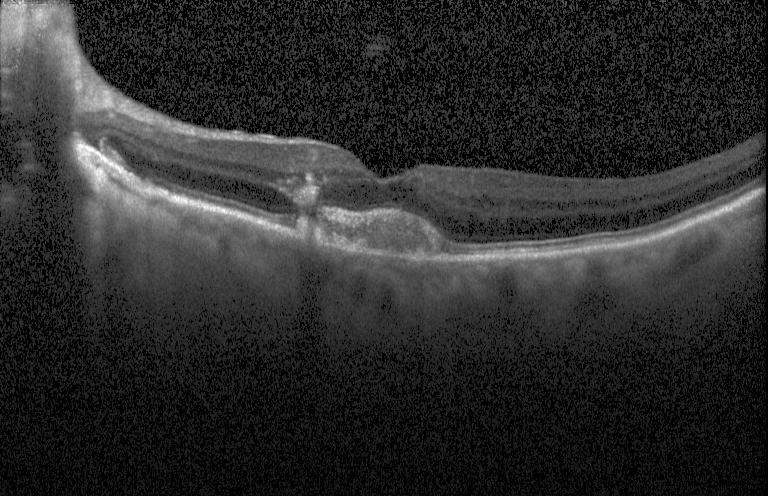 Assessment: a choroidal neovascular membrane.